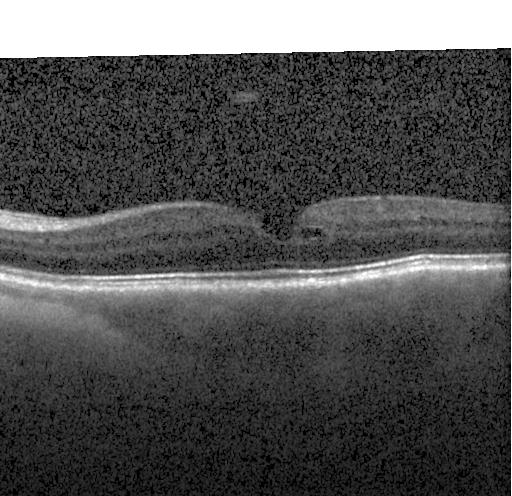

Optical coherence tomography scan. Macular OCT: diabetic macular edema (DME).